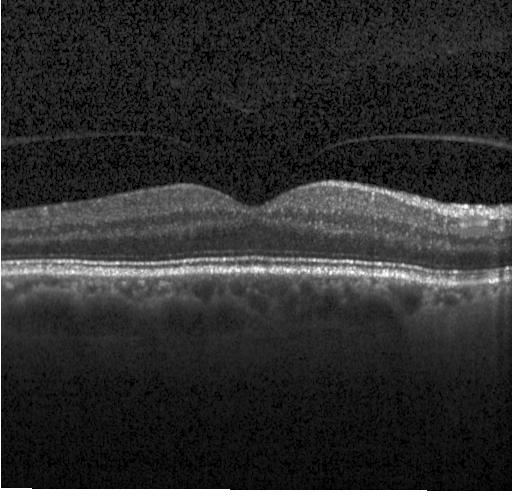

Retinal OCT cross-section.
This B-scan demonstrates no evidence of CNV, DME, or drusen.